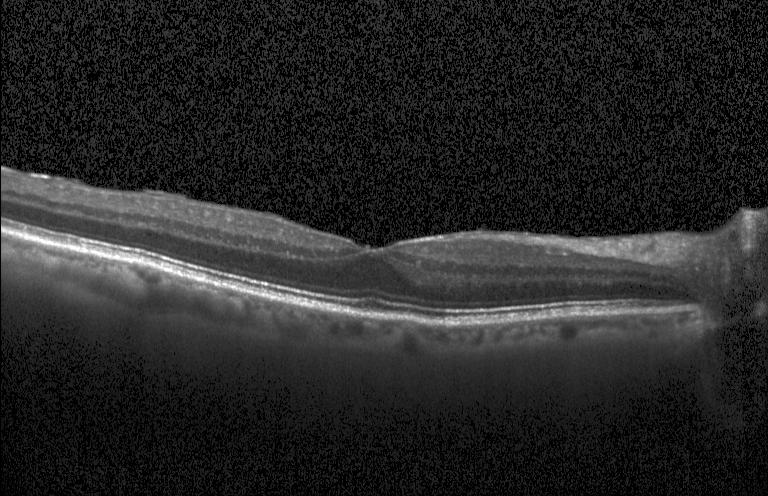
Spectral-domain OCT · instrument: Heidelberg Spectralis · horizontal scan through the fovea · retinal OCT cross-section. Finding: neither choroidal neovascularization, diabetic macular edema, nor drusen.